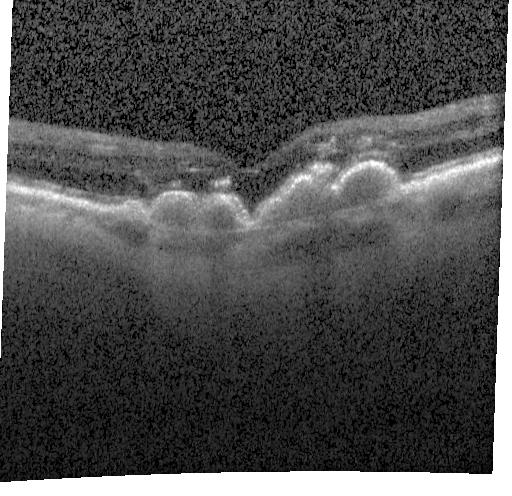
Centered on the fovea, OCT line scan, acquired on a Heidelberg Spectralis — Dx: a choroidal neovascular membrane.